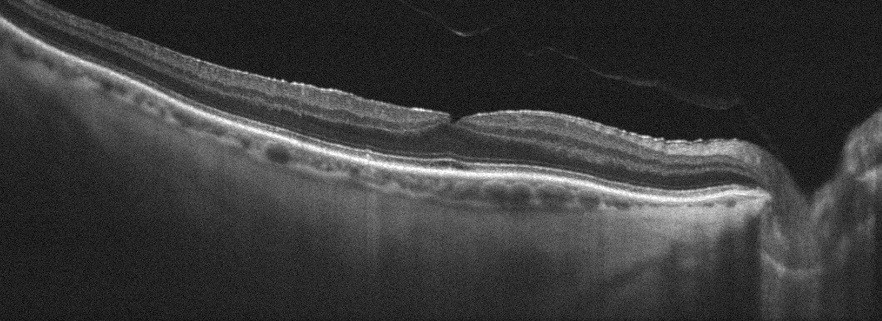

Through the macula. OCT B-scan — Epiretinal membrane.